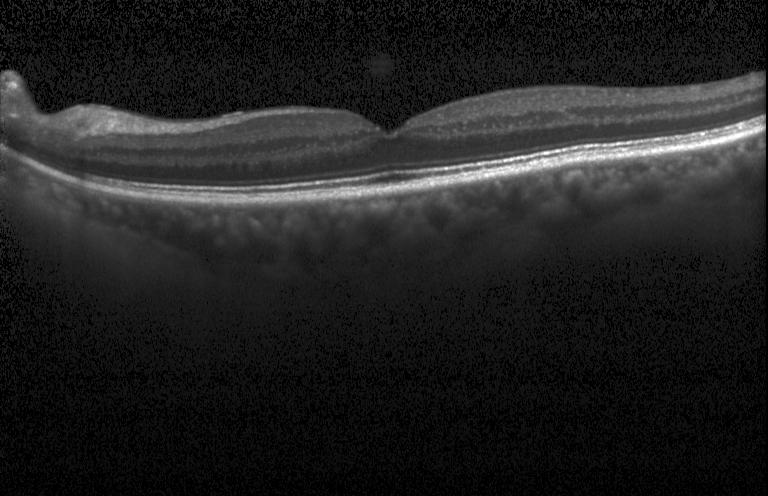 SD-OCT; macular scan; OCT B-scan — Impression: neither choroidal neovascularization, diabetic macular edema, nor drusen.